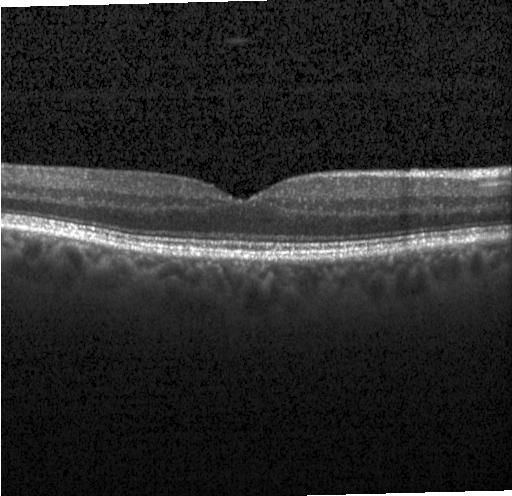 Dx: no CNV, DME, or drusen.